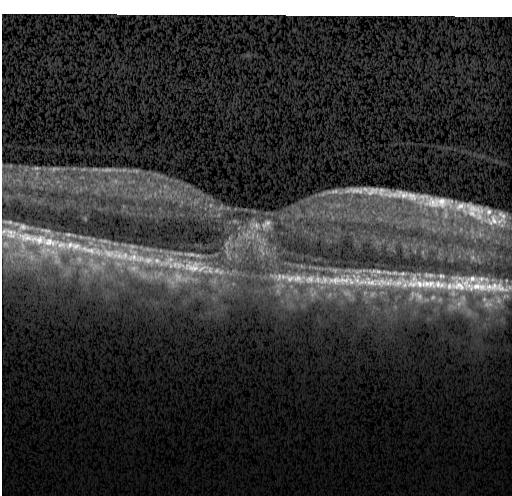 OCT line scan, centered on the fovea, Heidelberg Spectralis — Macular OCT: a choroidal neovascular membrane.